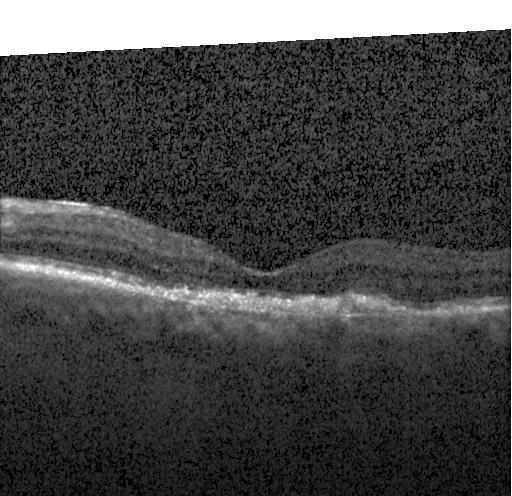 Through the macula. Heidelberg Spectralis. Optical coherence tomography B-scan.
Diagnosis: a choroidal neovascular membrane.